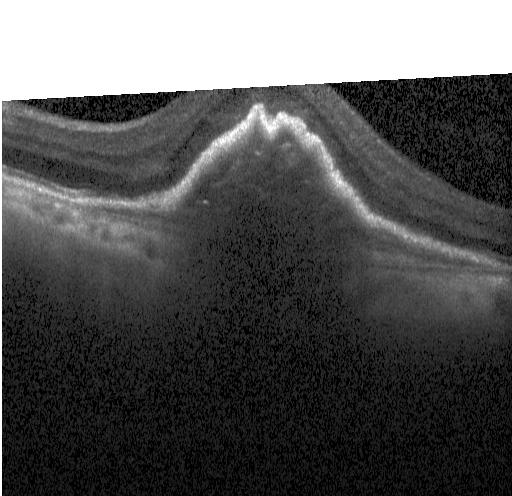 OCT line scan
Dx: a choroidal neovascular membrane.